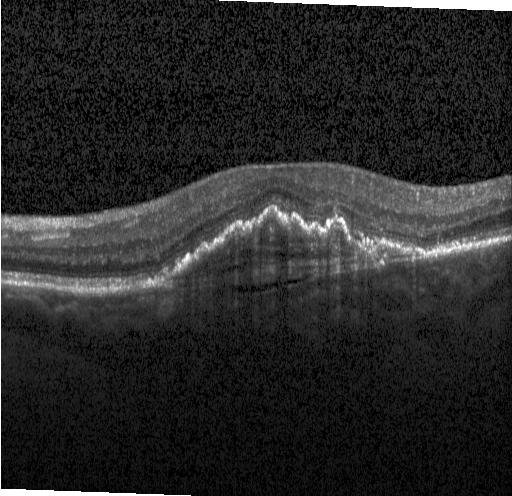
Retinal OCT cross-section showing a choroidal neovascular membrane.